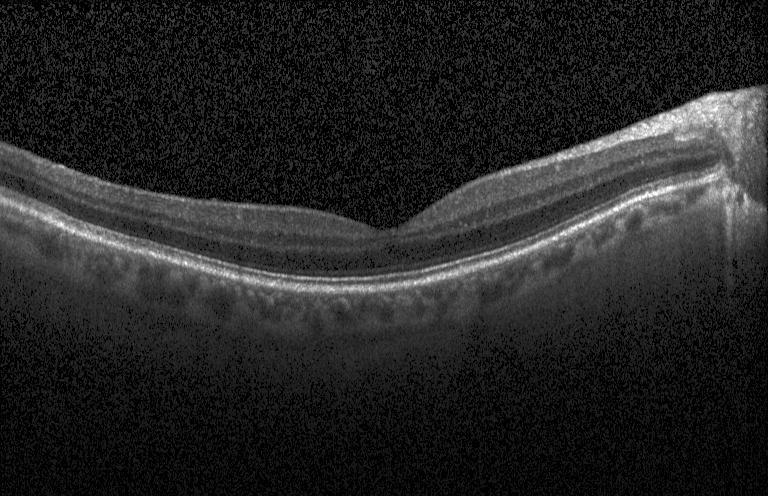

OCT line scan — Finding: no choroidal neovascularization, no diabetic macular edema, and no drusen.